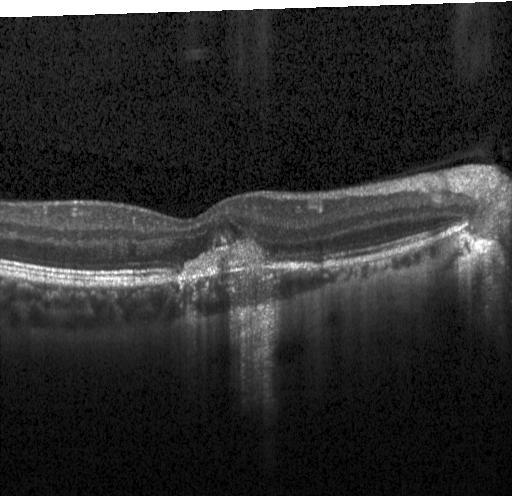 OCT B-scan — OCT finding: a choroidal neovascular membrane.